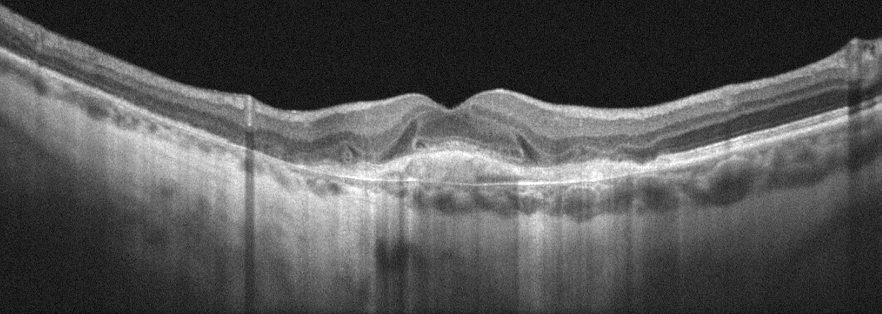

Diagnosis: age-related macular degeneration.